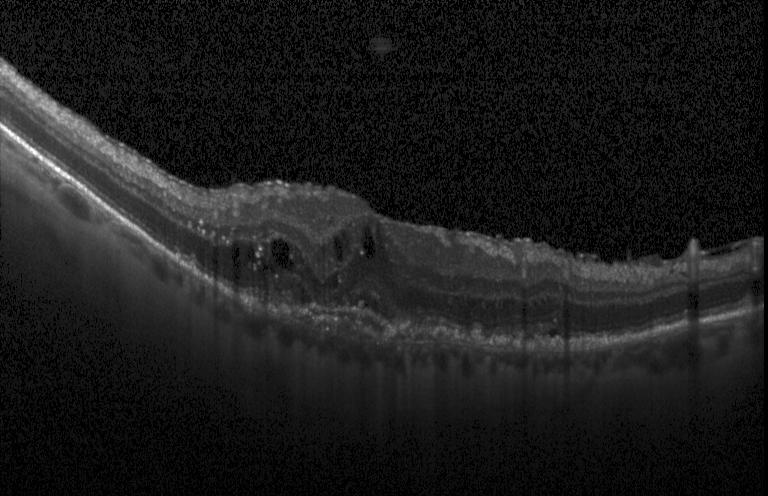
Spectral-domain OCT. Retinal OCT cross-section. Fovea-centered. Instrument: Heidelberg Spectralis — Impression: a choroidal neovascular membrane.